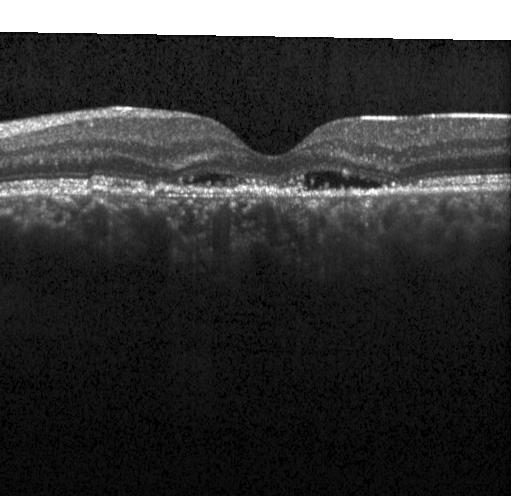

Finding: CNV.